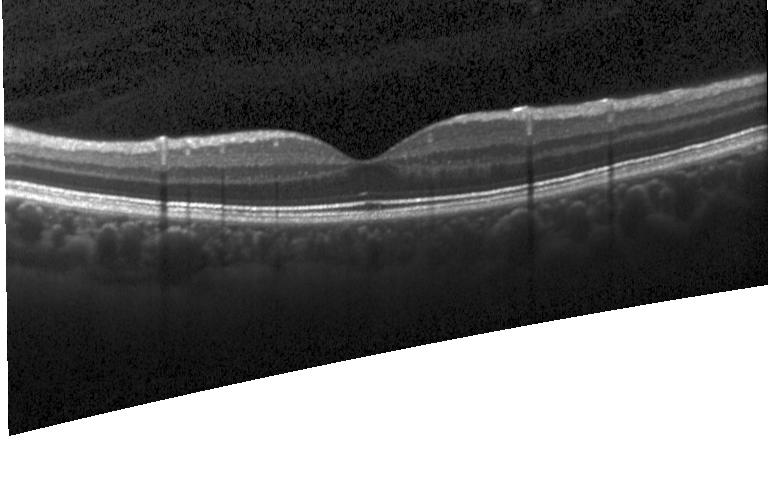

Optical coherence tomography scan. Spectral-domain OCT
Diagnosis: neither CNV, DME, nor drusen.